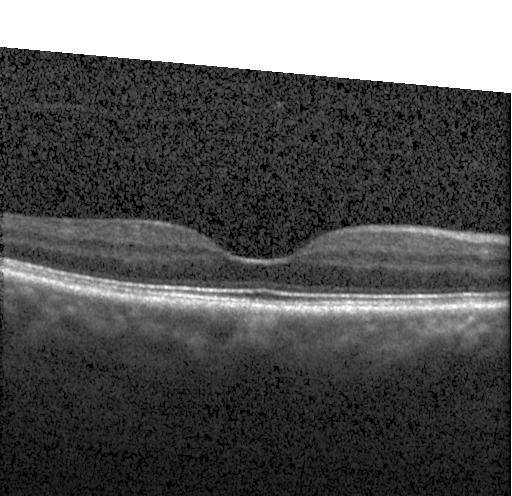 Impression: no evidence of CNV, DME, or drusen.